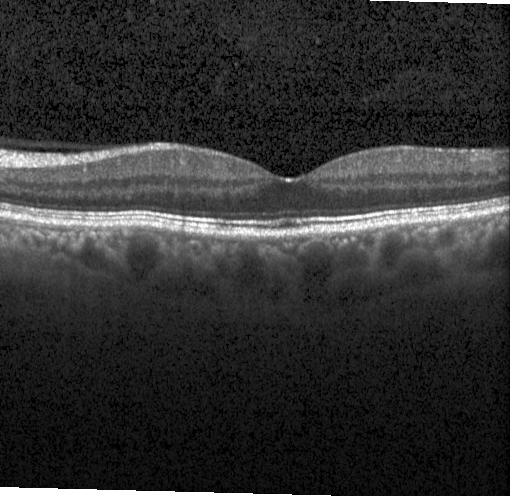
Retinal OCT cross-section showing no CNV, no DME, and no drusen.